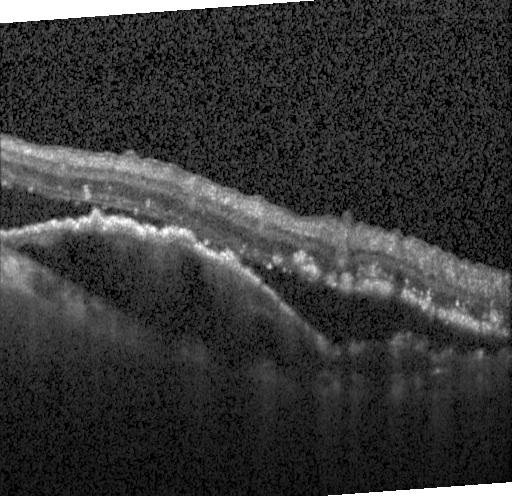

Diagnosis: a choroidal neovascular membrane.